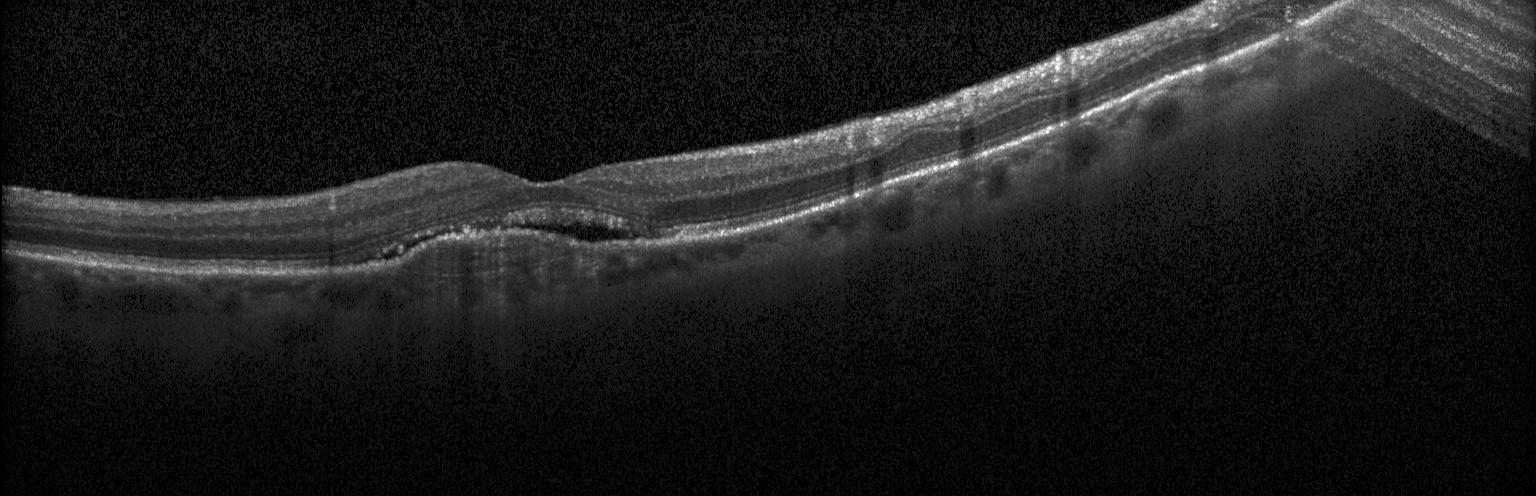 Spectral-domain optical coherence tomography. Instrument: Heidelberg Spectralis. Fovea-centered. OCT B-scan. Diagnosis: CNV.